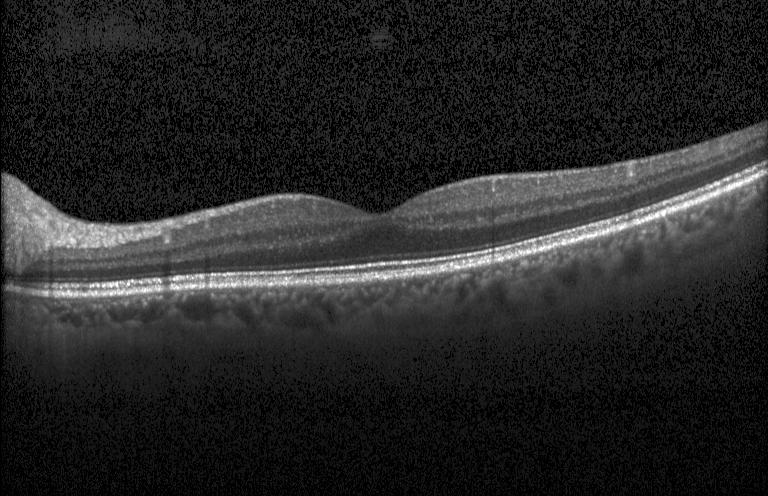
Optical coherence tomography scan. The scan shows no choroidal neovascularization, no diabetic macular edema, and no drusen.